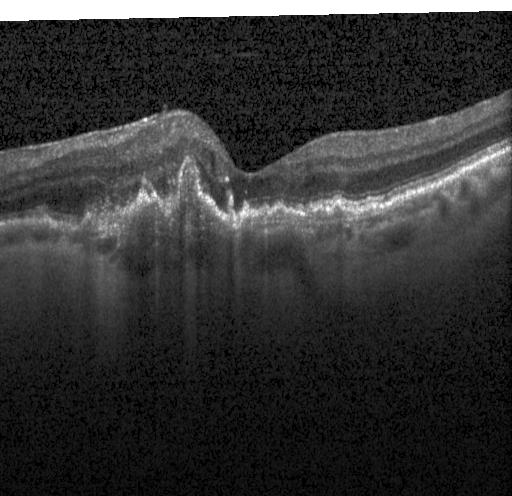

Optical coherence tomography scan — Diagnosis: a choroidal neovascular membrane.